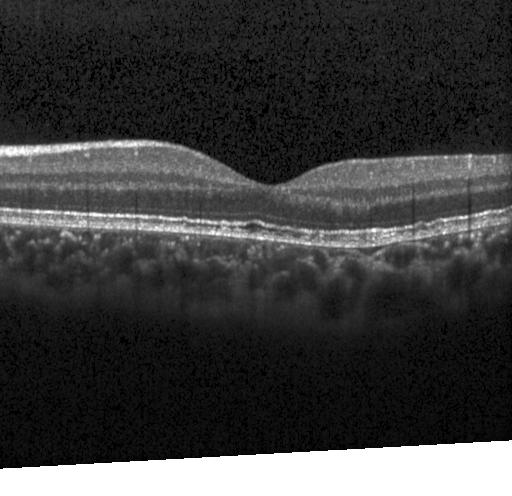 Finding: neither choroidal neovascularization, diabetic macular edema, nor drusen.